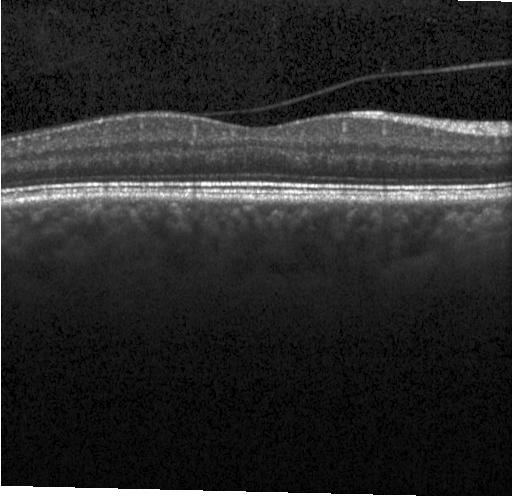
Diagnosis: no choroidal neovascularization, no diabetic macular edema, and no drusen.